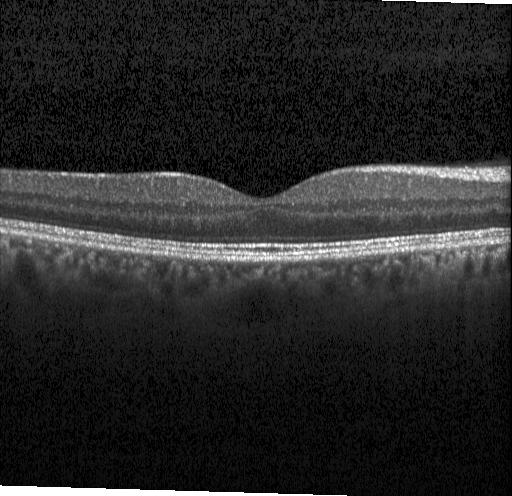 Dx: no choroidal neovascularization, no diabetic macular edema, and no drusen.